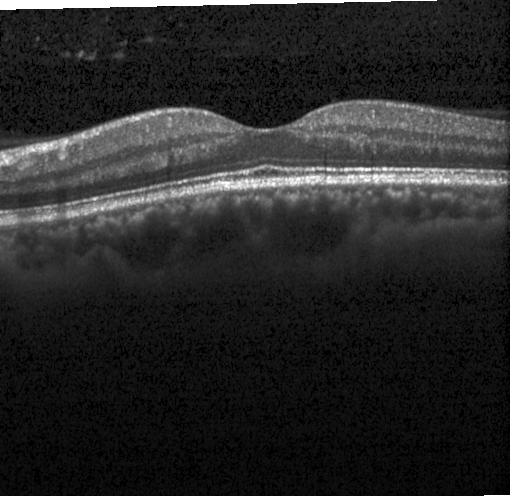 Optical coherence tomography scan — Diagnosis: neither choroidal neovascularization, diabetic macular edema, nor drusen.